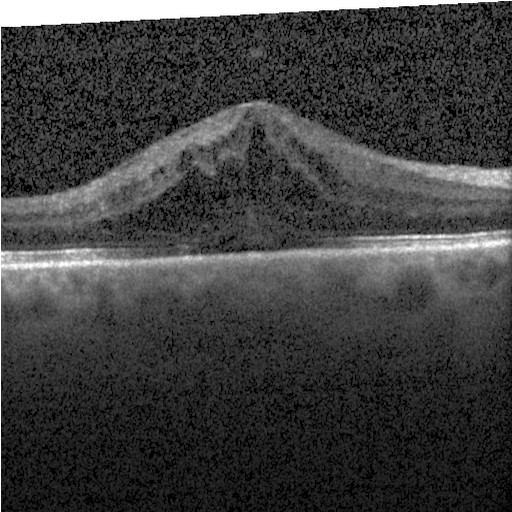 OCT finding: diabetic macular edema (DME).